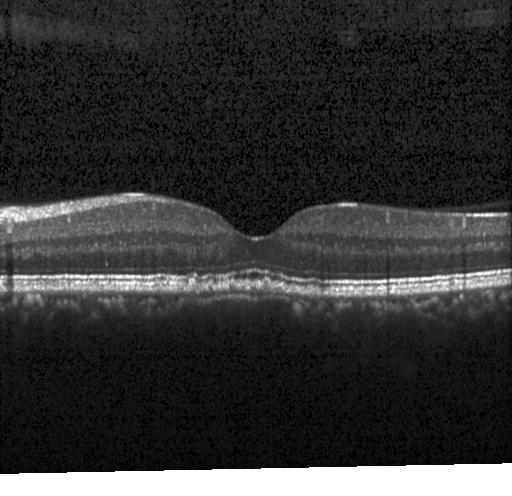 Spectral-domain OCT. OCT B-scan
Impression: sub-RPE drusenoid deposits.